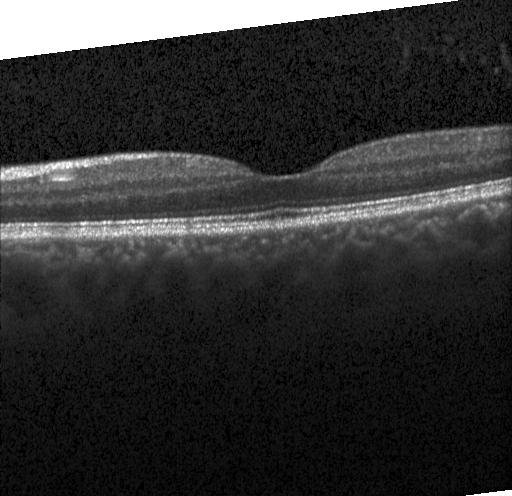 OCT finding: no choroidal neovascularization, diabetic macular edema, or drusen.